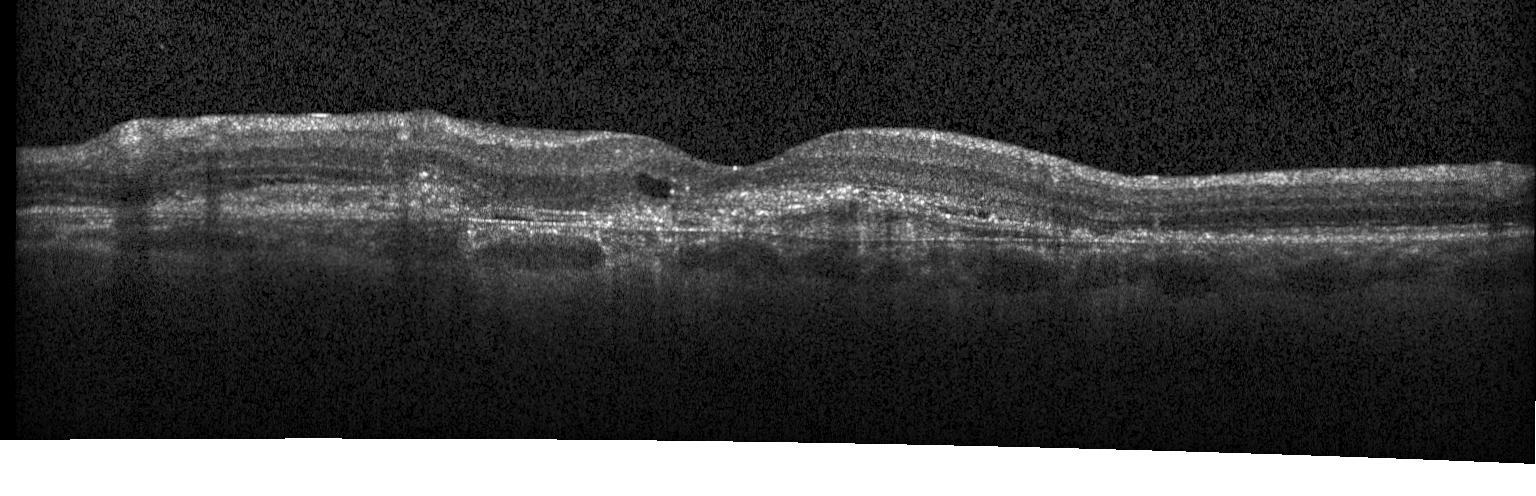

Macular OCT: choroidal neovascularization (CNV).